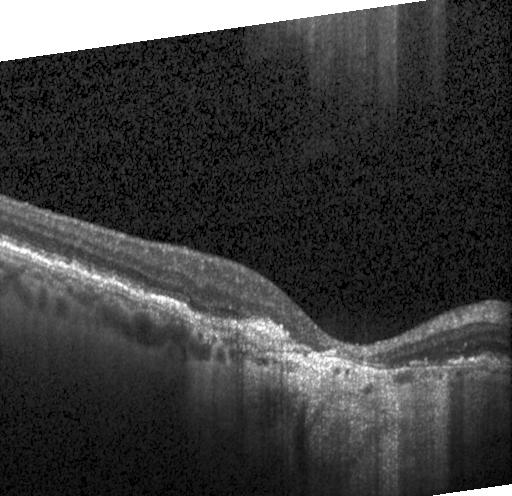 Impression: choroidal neovascularization (CNV).